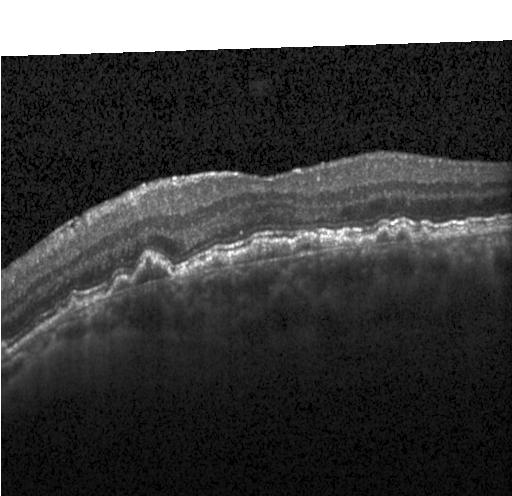 OCT B-scan · macular scan · spectral-domain optical coherence tomography — Assessment: a choroidal neovascular membrane.